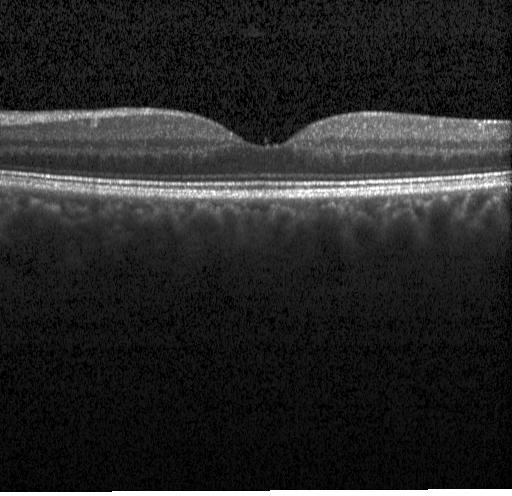
OCT line scan; acquired on a Heidelberg Spectralis.
Finding: no choroidal neovascularization, diabetic macular edema, or drusen.